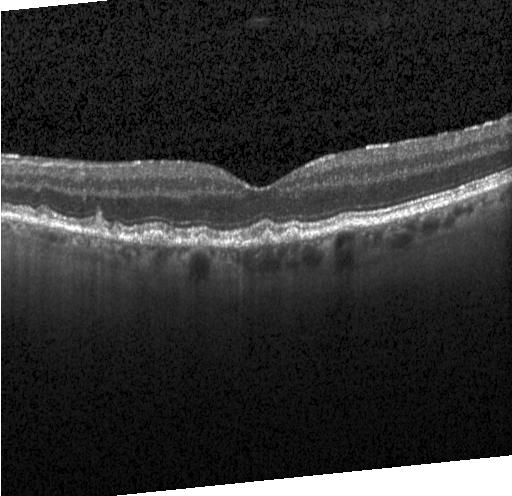

Dx: sub-RPE drusenoid deposits.